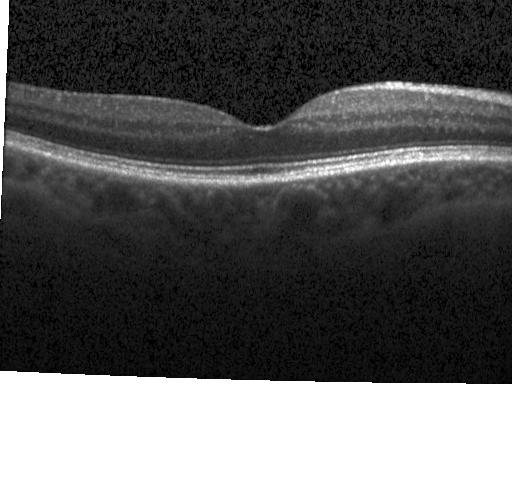 Spectral-domain OCT B-scan: no evidence of choroidal neovascularization, diabetic macular edema, or drusen.